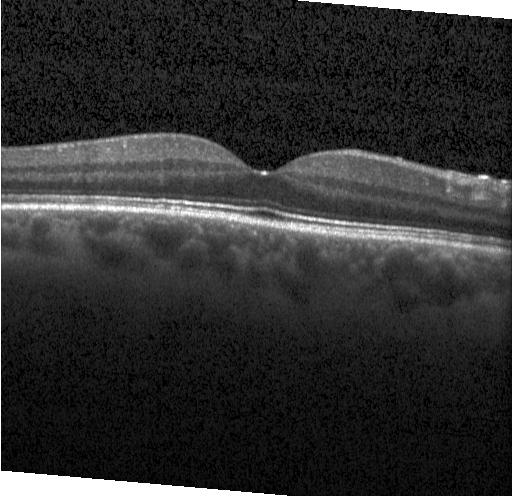 SD-OCT · acquired on a Heidelberg Spectralis · optical coherence tomography B-scan · macular scan. Finding: neither CNV, DME, nor drusen.